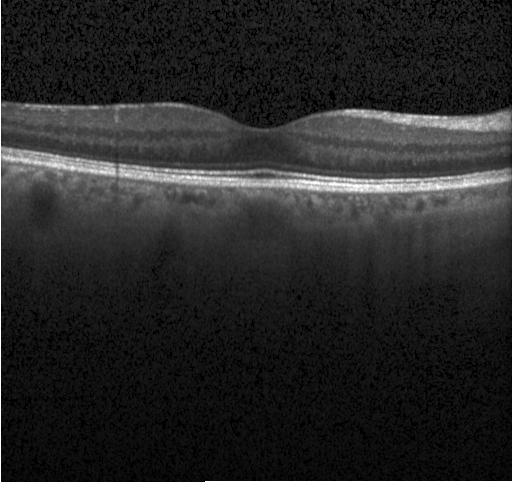
Retinal OCT B-scan. No CNV, no DME, and no drusen.